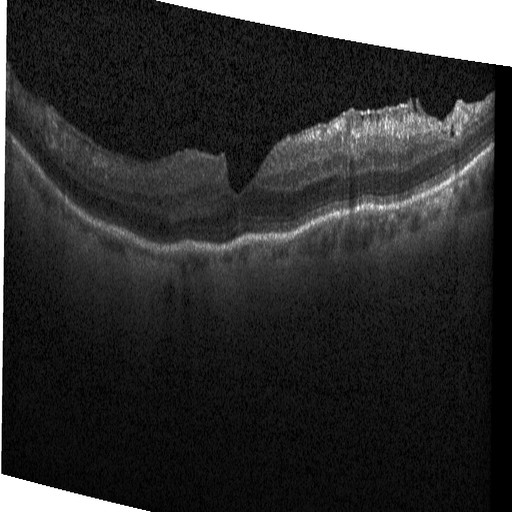 Diagnosis: diabetic macular edema.